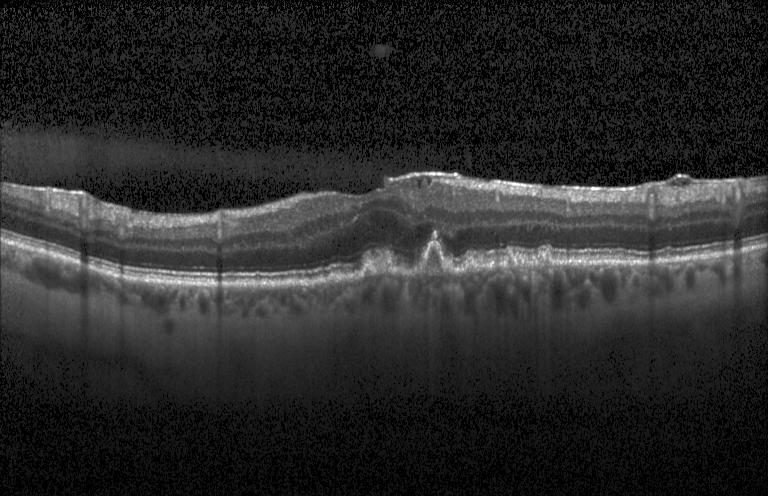 OCT line scan · spectral-domain OCT · instrument: Heidelberg Spectralis
Macular OCT: drusen.